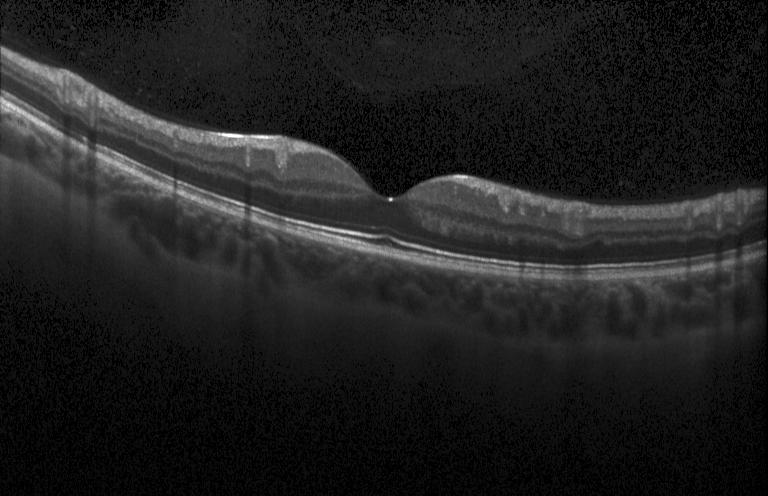 Spectral-domain optical coherence tomography. Instrument: Heidelberg Spectralis. Fovea-centered. Retinal OCT cross-section.
Dx: no choroidal neovascularization, no diabetic macular edema, and no drusen.